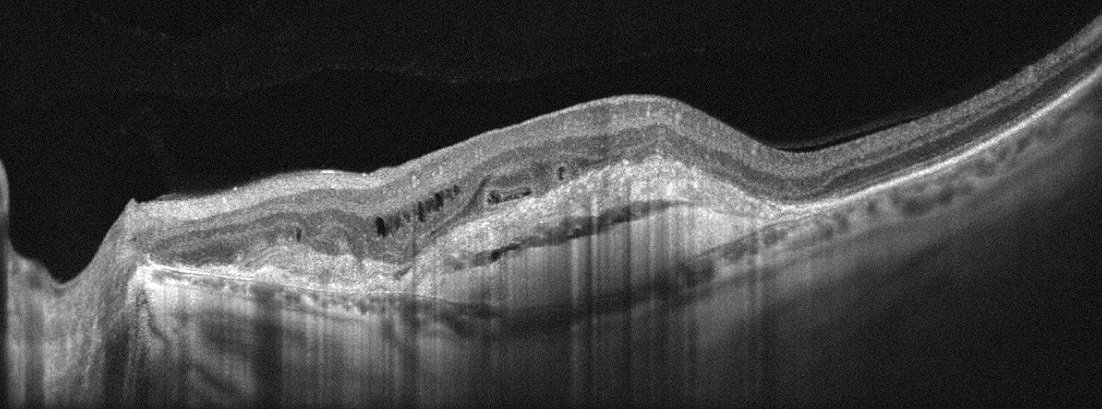 OCT scan showing AMD.